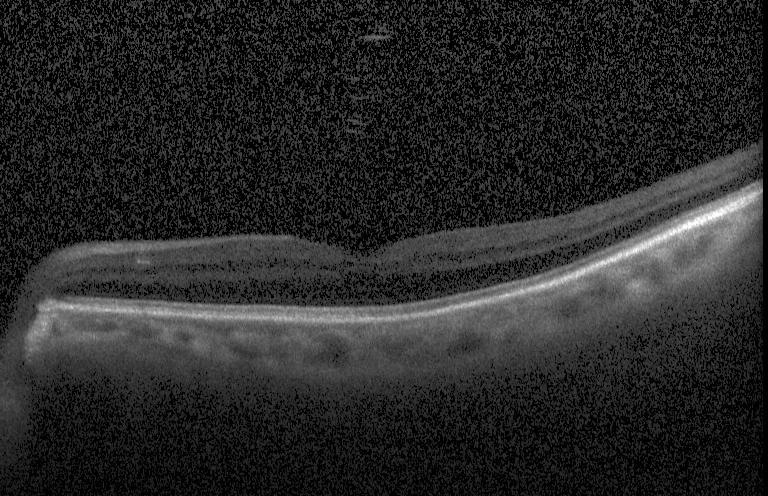
Spectral-domain OCT; OCT line scan
Impression: no choroidal neovascularization, no diabetic macular edema, and no drusen.